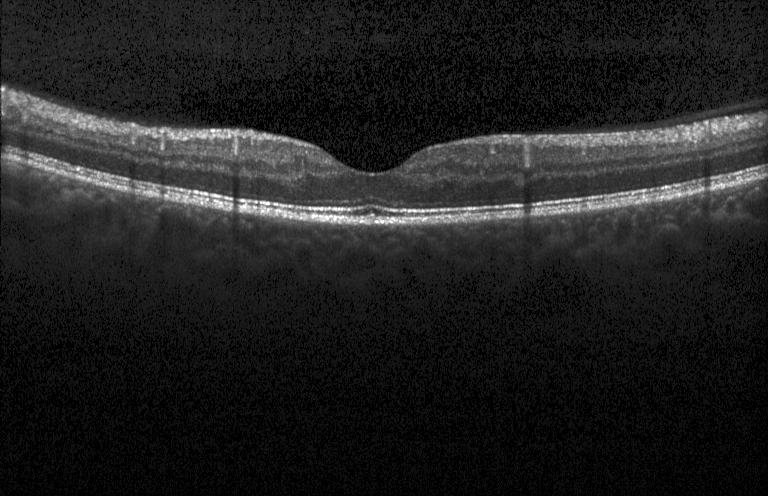

Dx: no choroidal neovascularization, diabetic macular edema, or drusen.